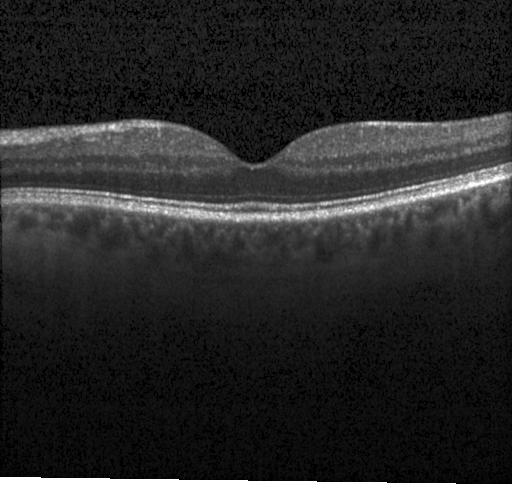 OCT finding: no choroidal neovascularization, diabetic macular edema, or drusen.